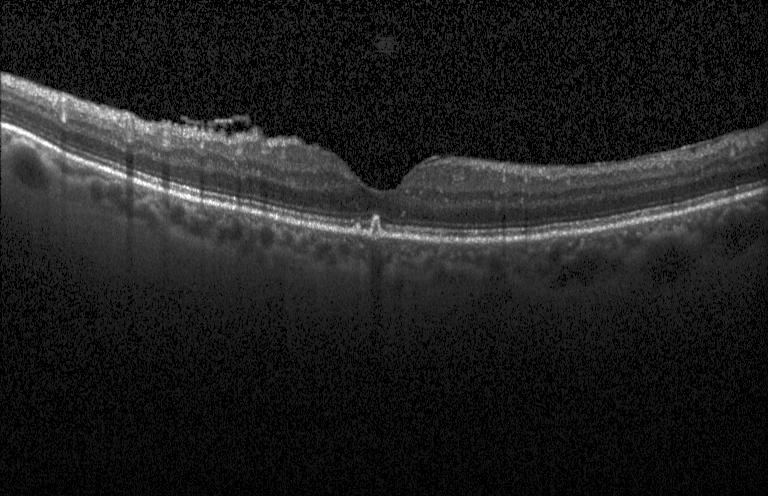 Spectral-domain OCT B-scan: multiple drusen.